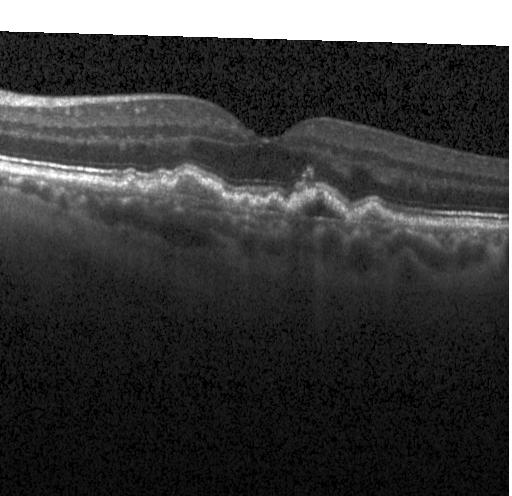
OCT B-scan, spectral-domain optical coherence tomography, through the macula, acquired on a Heidelberg Spectralis — The scan shows drusen.